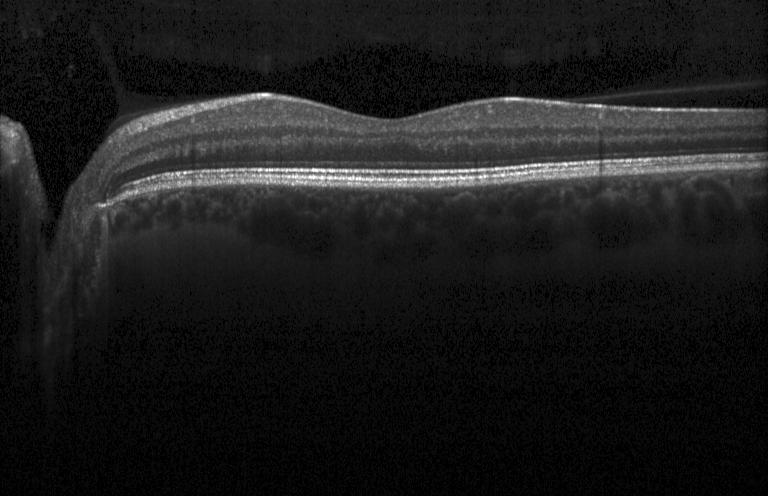

Neither CNV, DME, nor drusen.